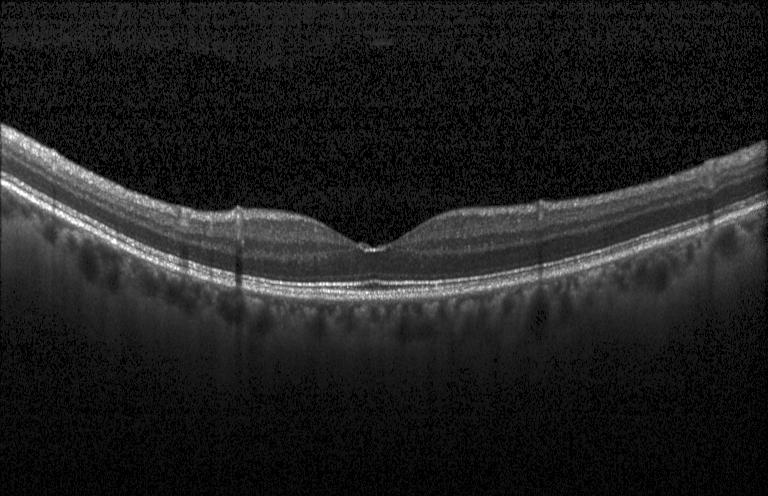
Neither choroidal neovascularization, diabetic macular edema, nor drusen.